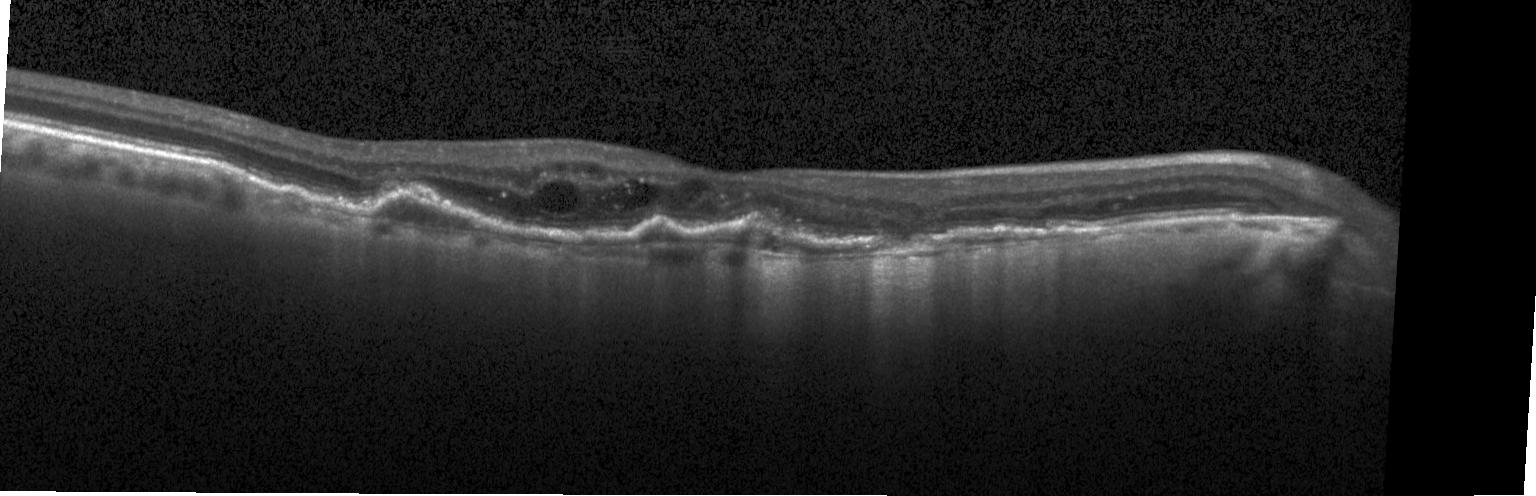 Macular OCT demonstrating a choroidal neovascular membrane.